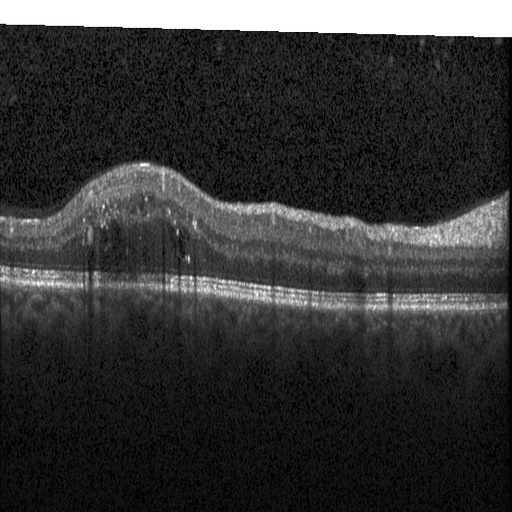
Optical coherence tomography B-scan; spectral-domain OCT; macular scan; acquired on a Heidelberg Spectralis.
Diagnosis: diabetic macular edema.